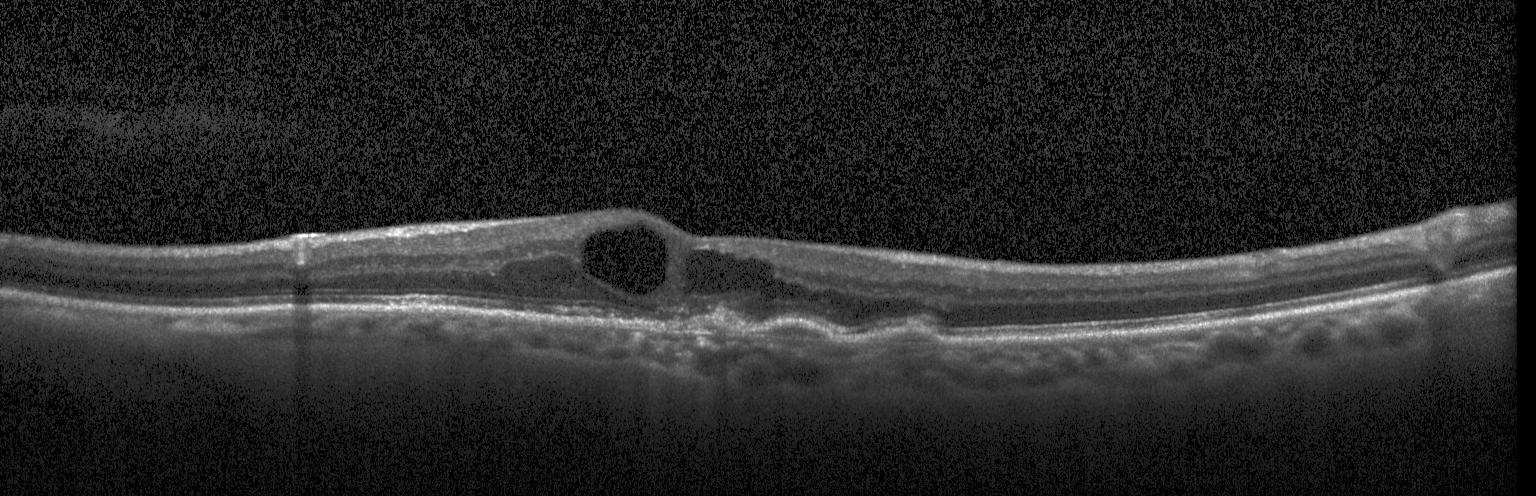

Impression: a choroidal neovascular membrane.